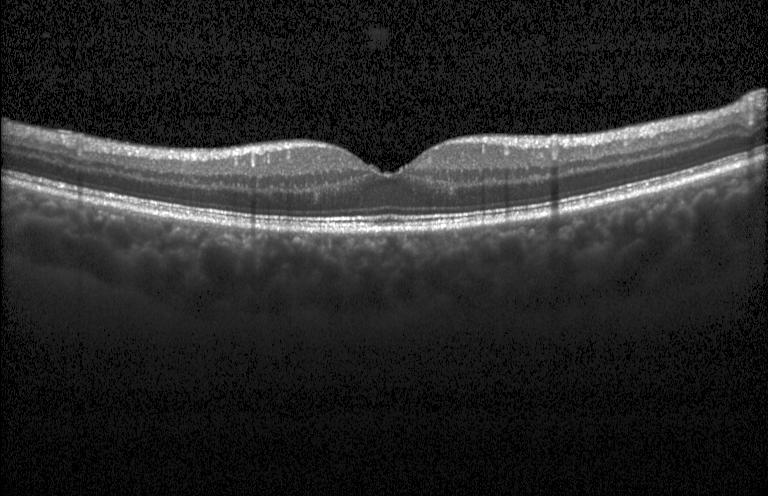

Finding: neither choroidal neovascularization, diabetic macular edema, nor drusen.